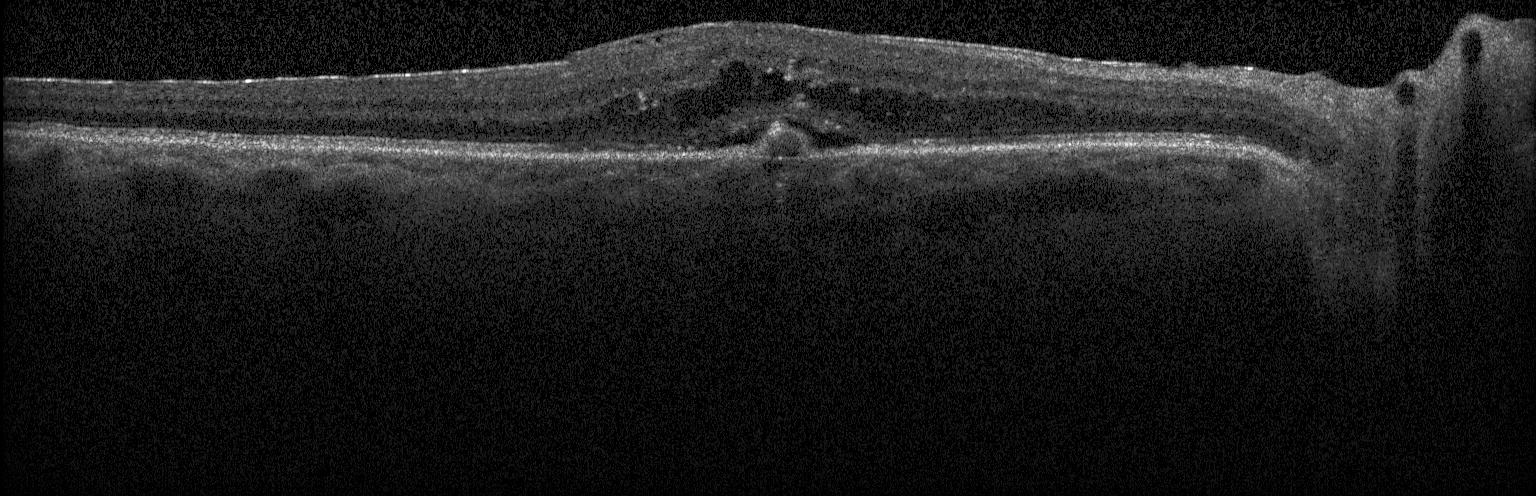 Macular OCT: a choroidal neovascular membrane.